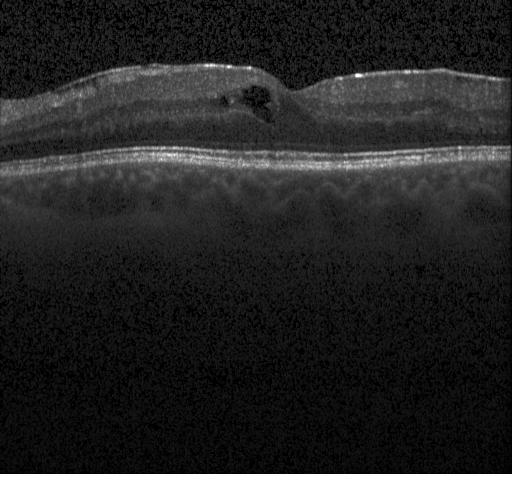

OCT B-scan showing diabetic macular edema.